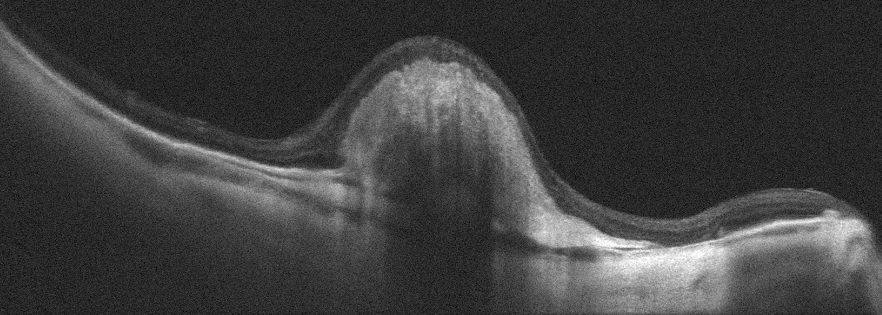
OCT line scan. Oculus dexter
OCT finding: age-related macular degeneration.